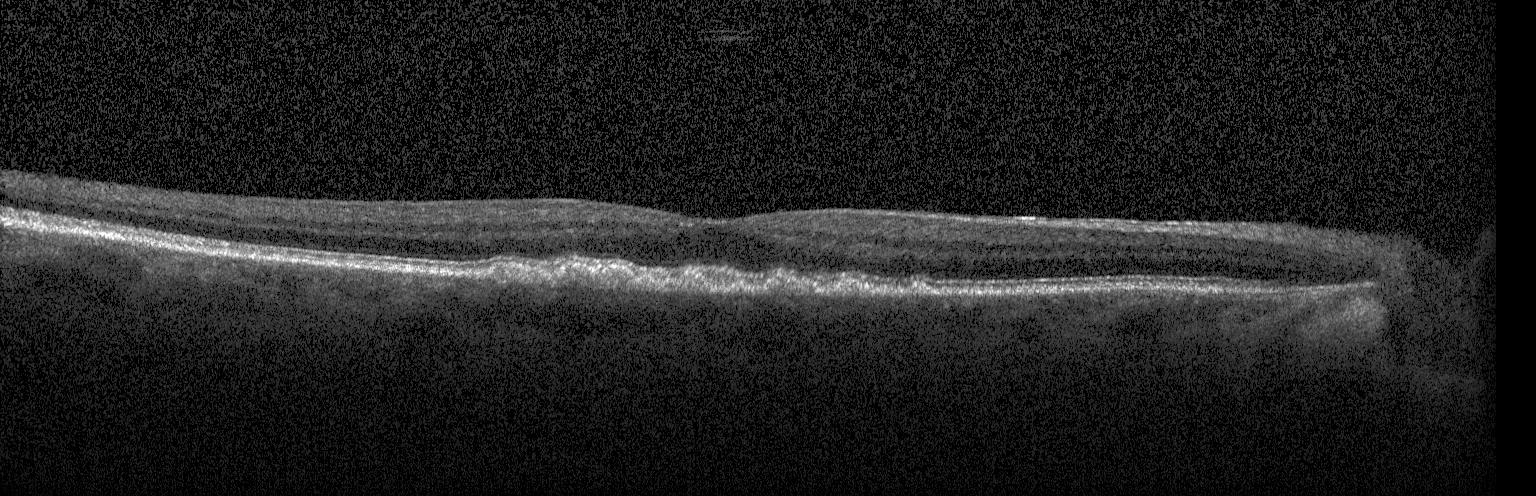

Centered on the fovea · retinal OCT cross-section — Assessment: multiple drusen.